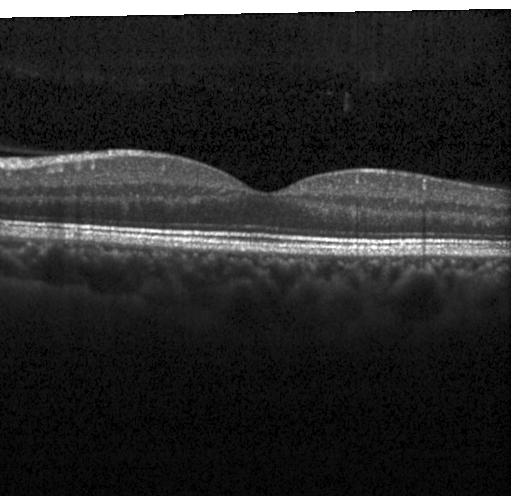 Macular scan; optical coherence tomography B-scan; spectral-domain OCT
Dx: neither choroidal neovascularization, diabetic macular edema, nor drusen.